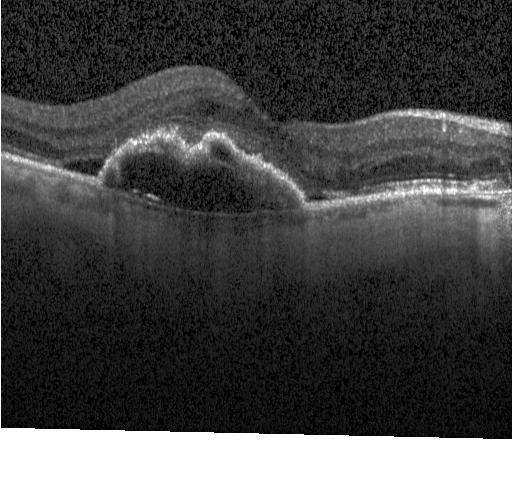 OCT B-scan.
OCT finding: a choroidal neovascular membrane.